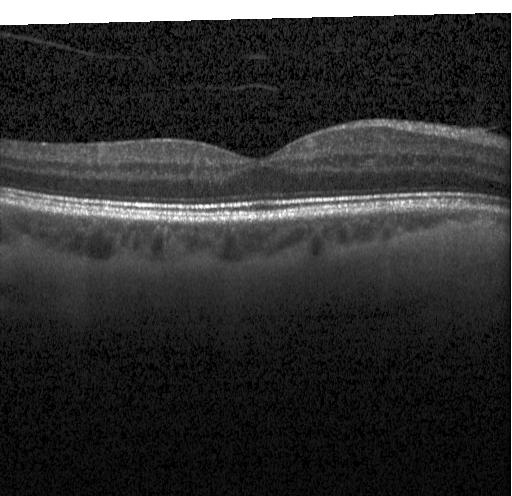

Optical coherence tomography scan · through the macula. This B-scan demonstrates no choroidal neovascularization, diabetic macular edema, or drusen.